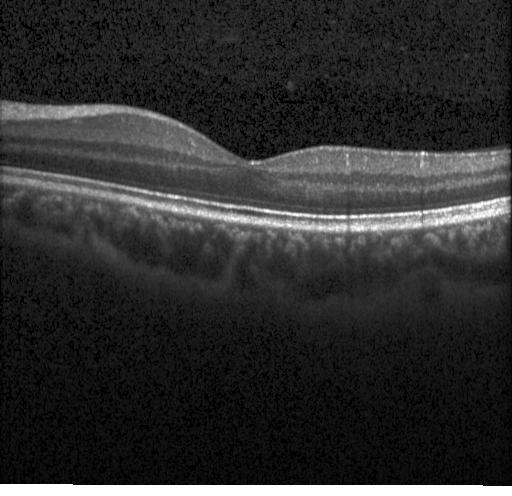 Through the macula · optical coherence tomography scan
No CNV, DME, or drusen.